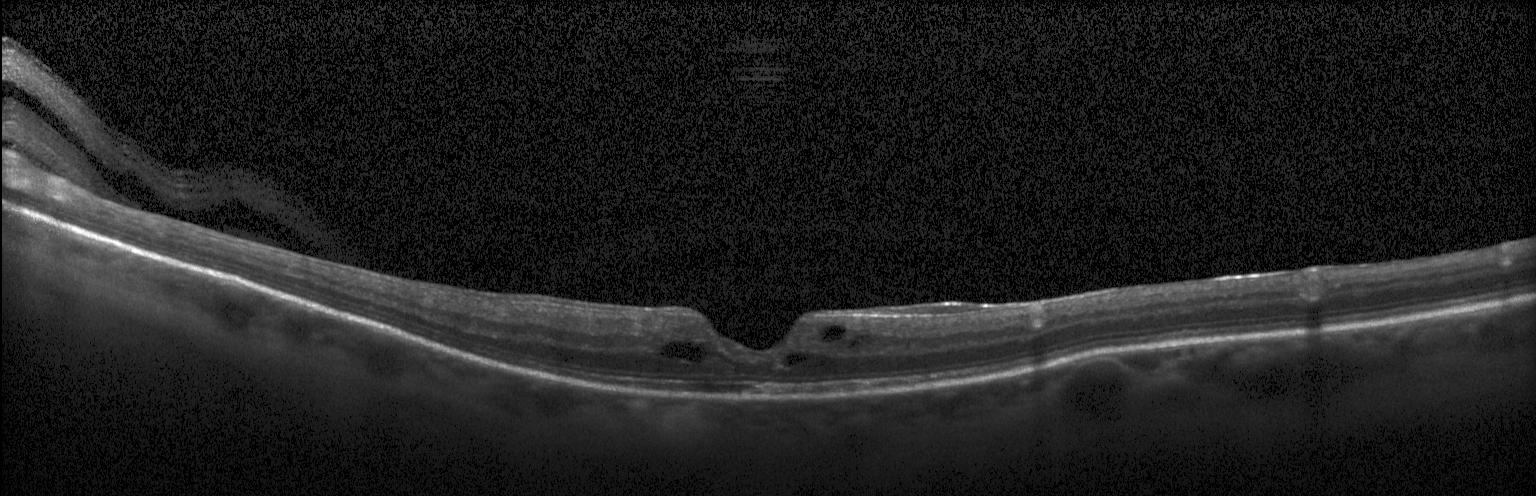
SD-OCT · retinal OCT cross-section · Heidelberg Spectralis · horizontal scan through the fovea. Diagnosis: diabetic macular edema.